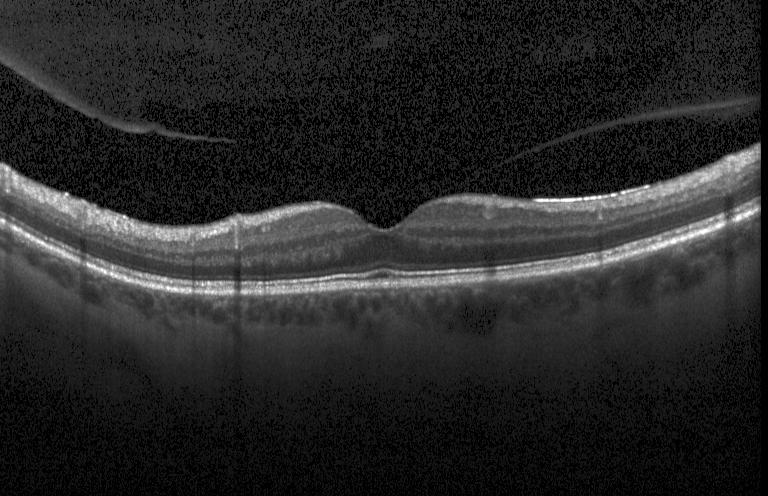 Through the macula, OCT B-scan — This B-scan demonstrates neither CNV, DME, nor drusen.